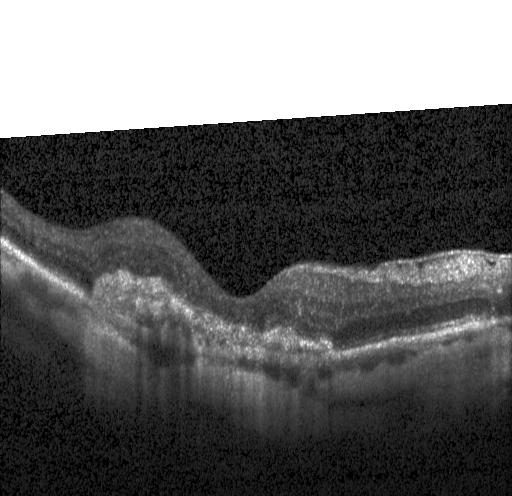

OCT B-scan. SD-OCT
Choroidal neovascularization (CNV).